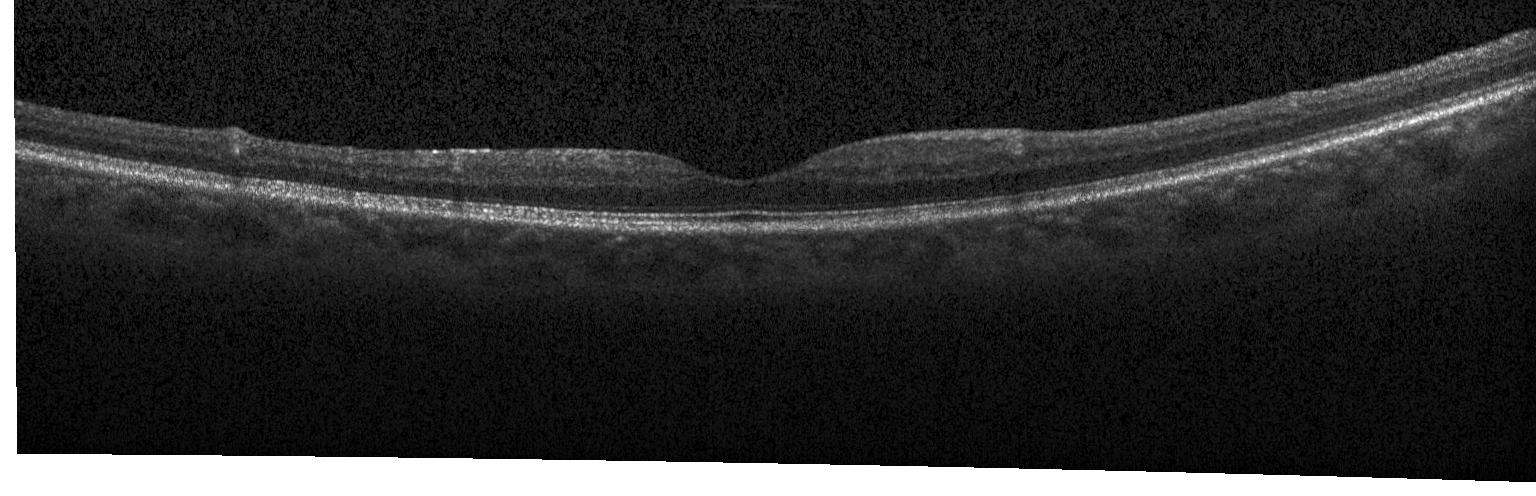
Diagnosis: no CNV, no DME, and no drusen.